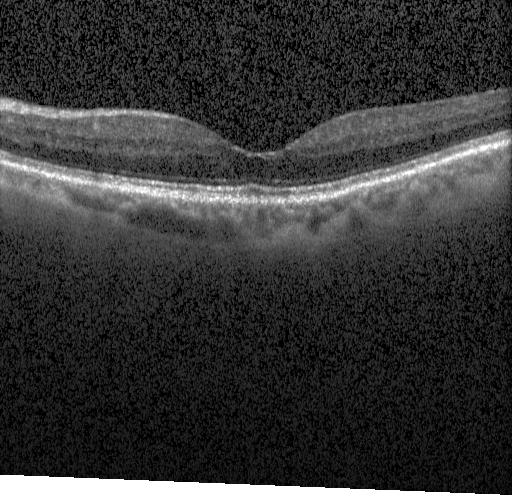
Finding: no CNV, no DME, and no drusen.